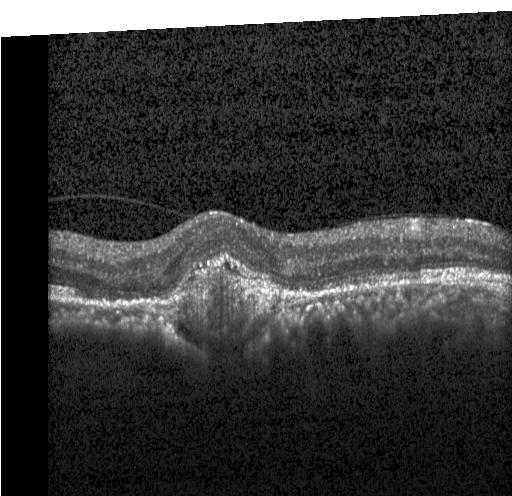
Acquired on a Heidelberg Spectralis · fovea-centered · SD-OCT · retinal OCT B-scan — Diagnosis: CNV.